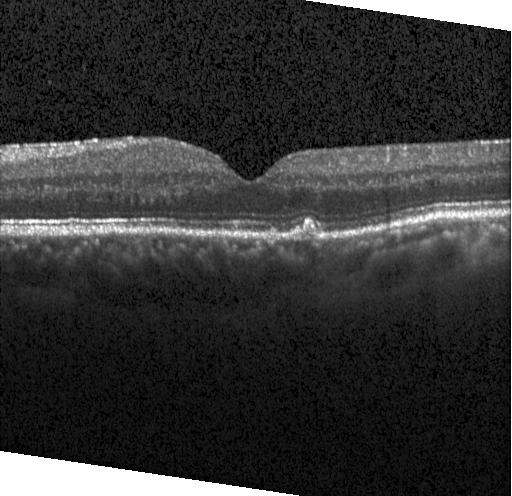

Heidelberg Spectralis, macular scan, retinal OCT B-scan. Finding: multiple drusen.